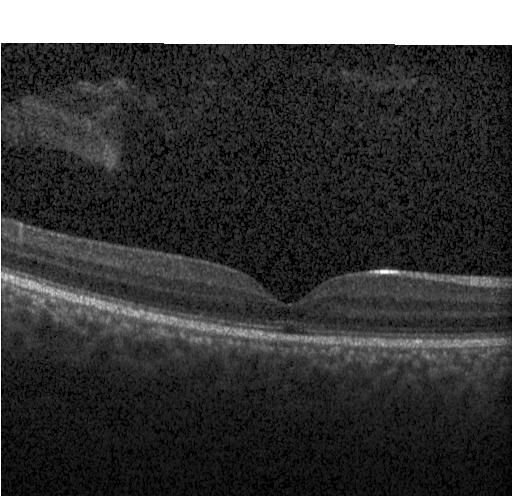

OCT line scan.
Macular OCT: no choroidal neovascularization, no diabetic macular edema, and no drusen.